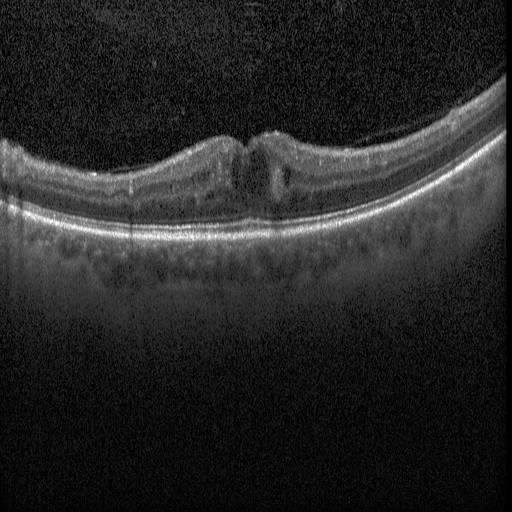

SD-OCT. OCT B-scan. The scan shows DME.